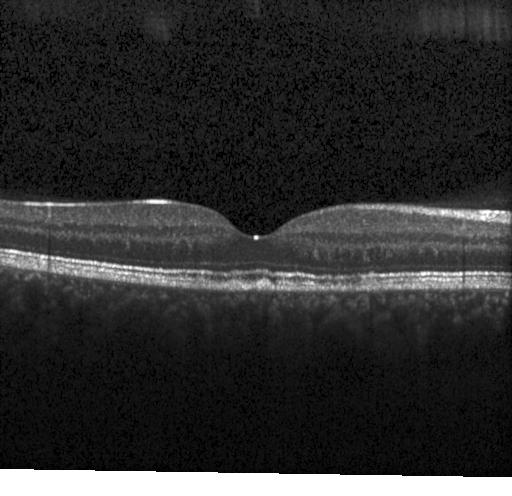 The scan shows multiple drusen.